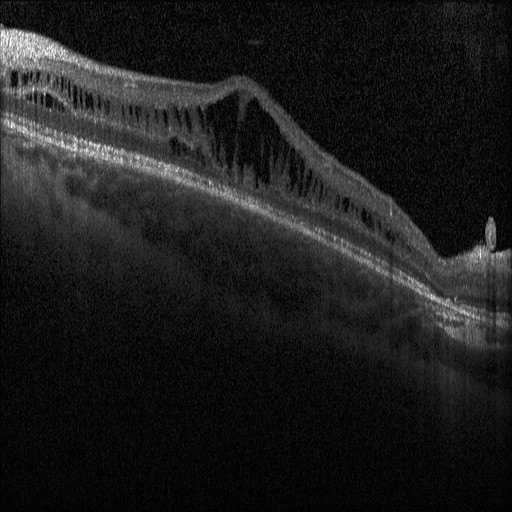
Retinal OCT B-scan, spectral-domain OCT, through the macula — Diabetic macular edema (DME).